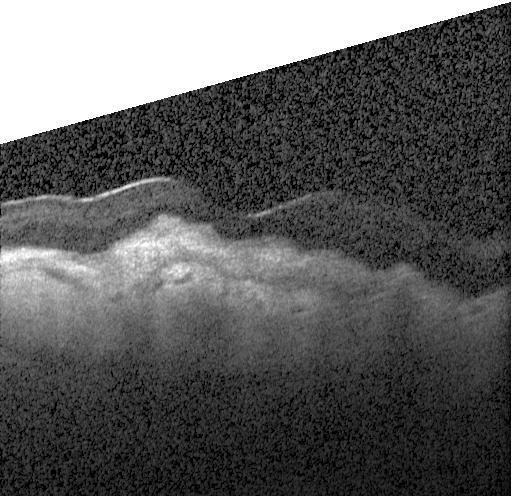
Assessment: a choroidal neovascular membrane.